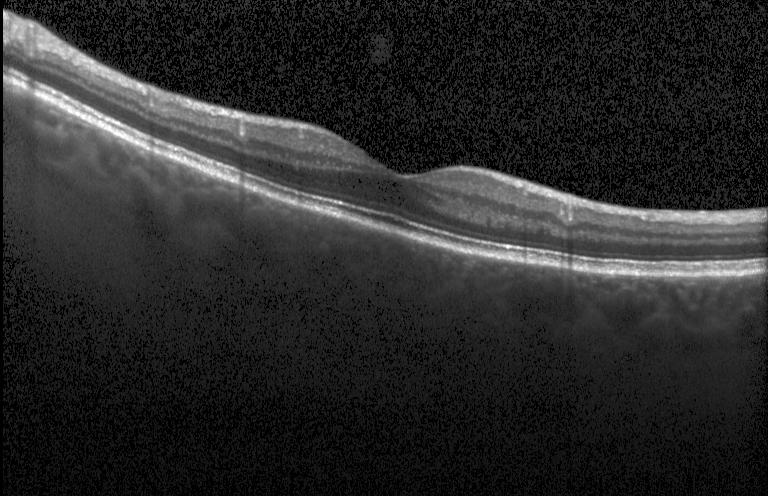
Dx: neither CNV, DME, nor drusen.